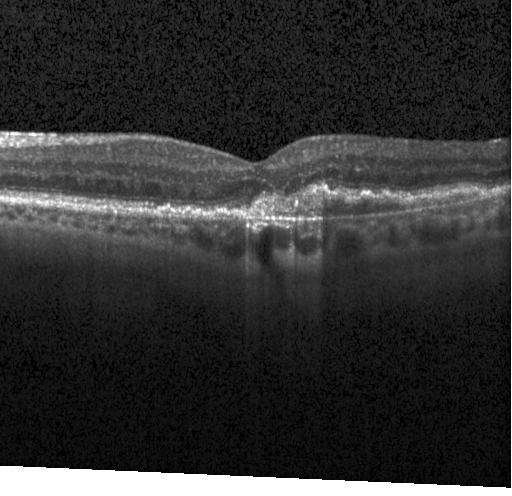

Retinal OCT cross-section showing a choroidal neovascular membrane.